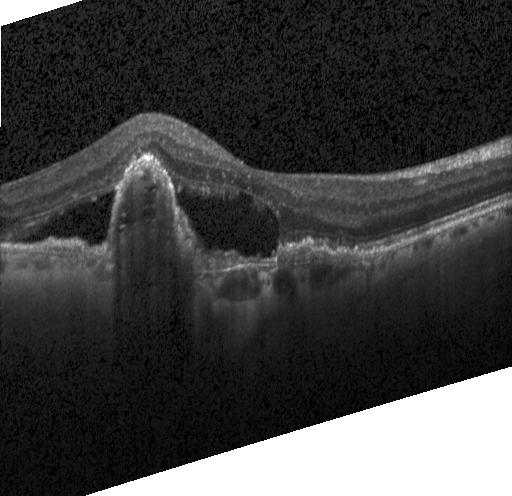
Spectral-domain OCT; OCT B-scan; centered on the fovea. The scan shows choroidal neovascularization (CNV).